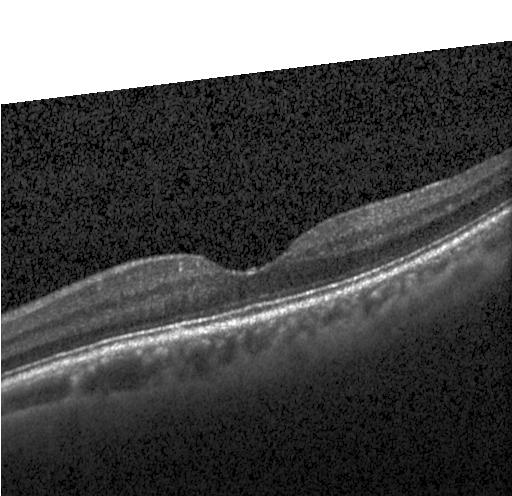 OCT scan showing no choroidal neovascularization, diabetic macular edema, or drusen.